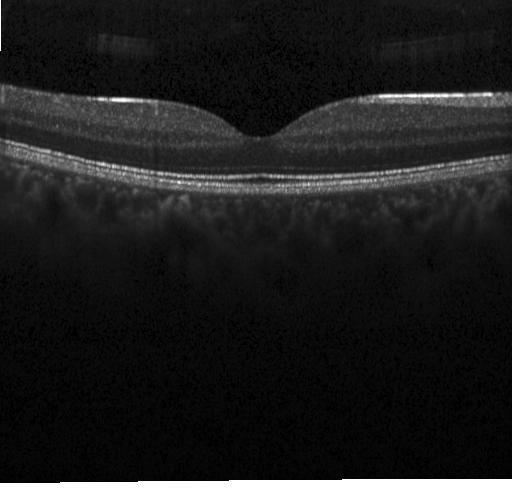

Impression: no CNV, no DME, and no drusen.